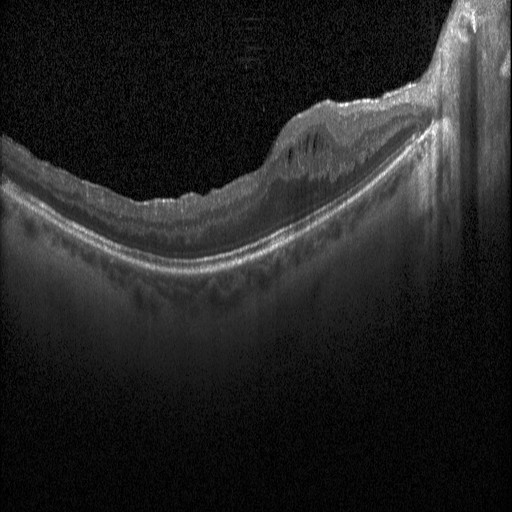

OCT scan showing diabetic macular edema.